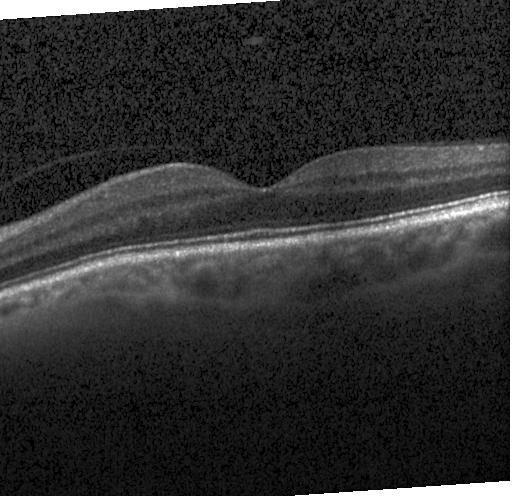
Diagnosis: no choroidal neovascularization, no diabetic macular edema, and no drusen.